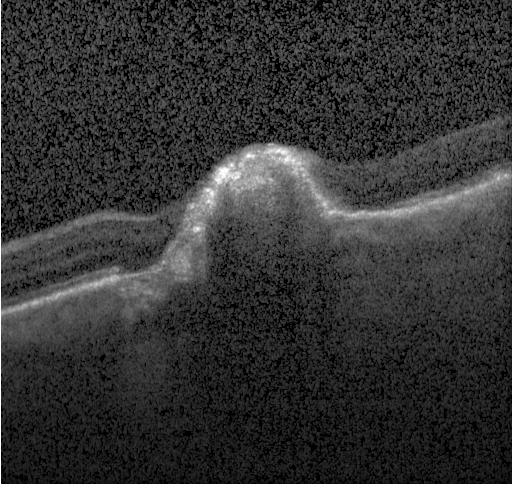

Retinal OCT cross-section — The scan shows a choroidal neovascular membrane.